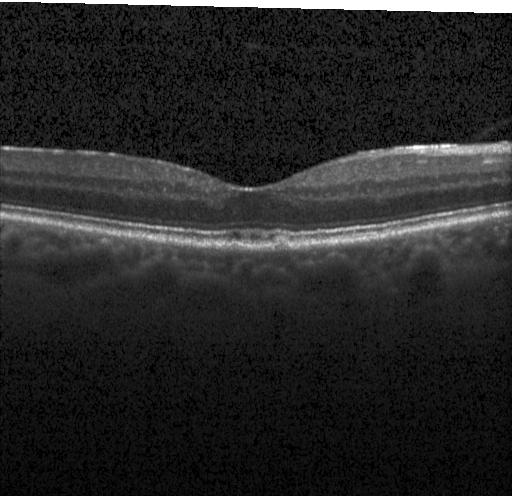 The scan shows sub-RPE drusenoid deposits.